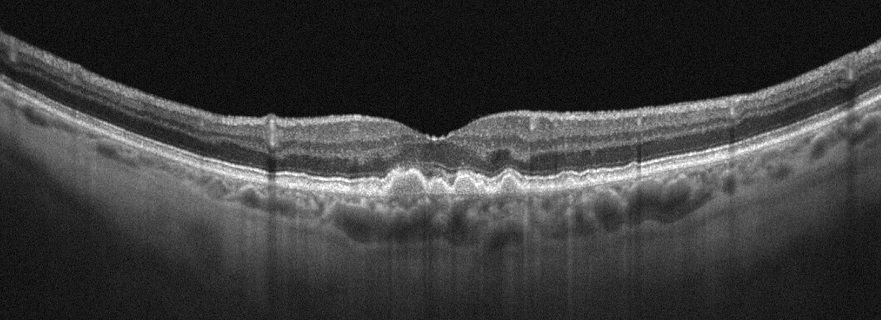 OCT B-scan.
Macular OCT: AMD.